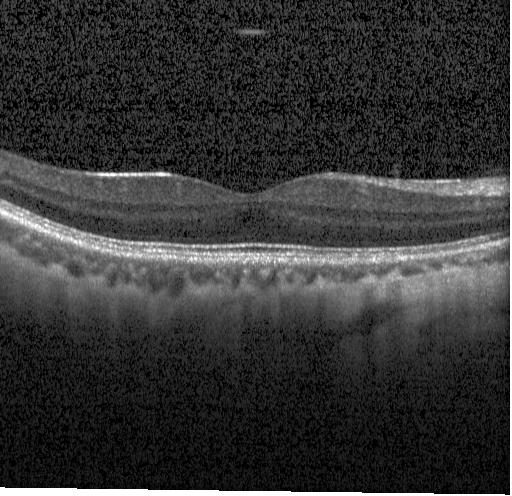

Centered on the fovea. OCT B-scan — Neither choroidal neovascularization, diabetic macular edema, nor drusen.